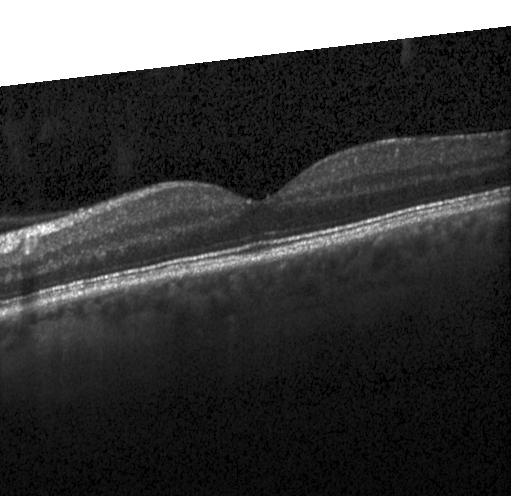
Heidelberg Spectralis; SD-OCT; OCT B-scan — Assessment: no choroidal neovascularization, diabetic macular edema, or drusen.